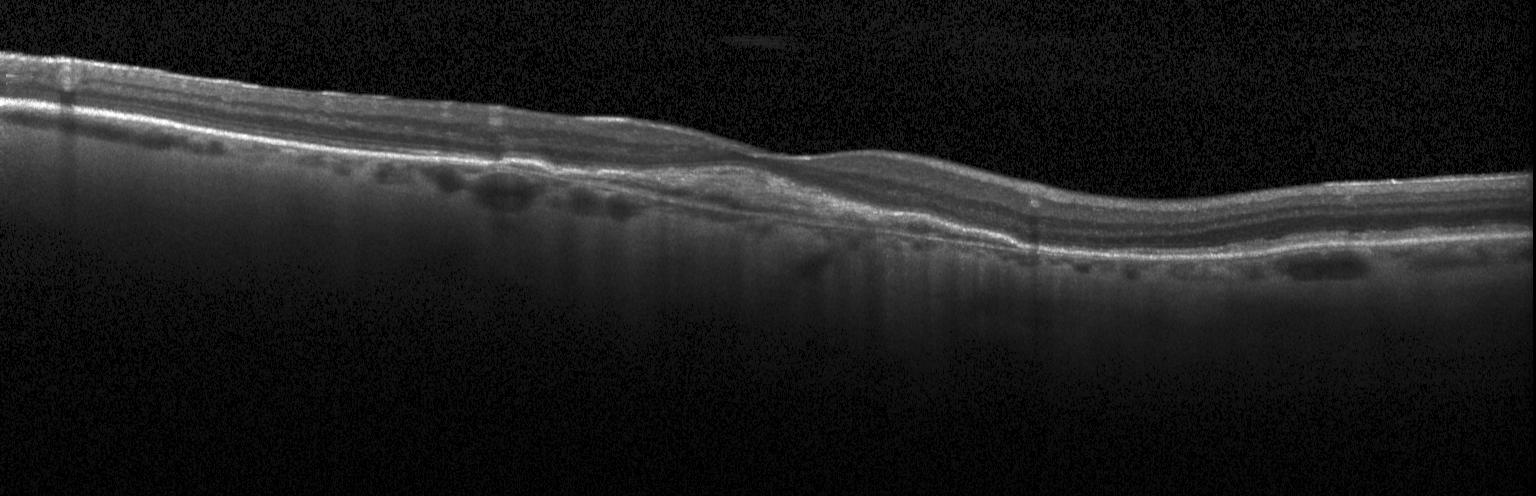

Retinal OCT cross-section showing a choroidal neovascular membrane.